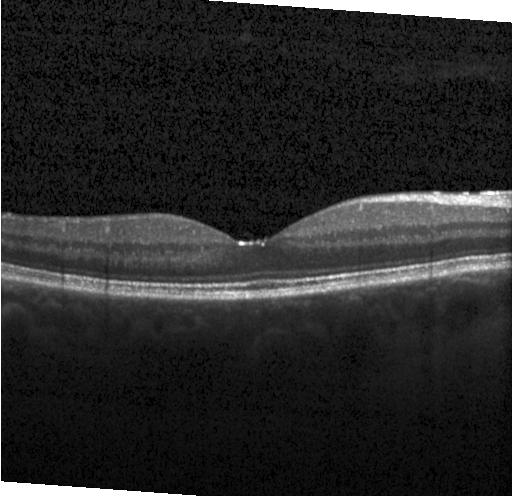

OCT B-scan, through the macula.
Diagnosis: no CNV, no DME, and no drusen.